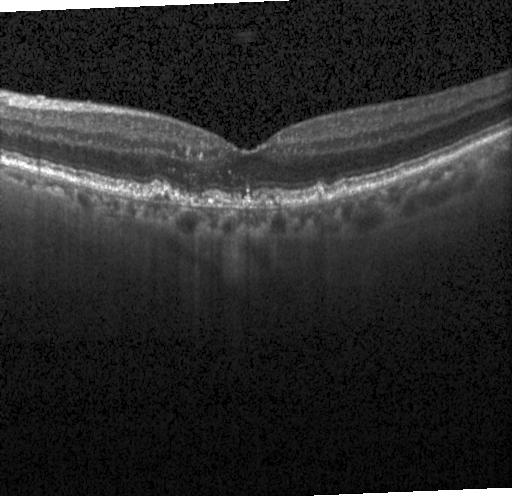
Spectral-domain OCT; Heidelberg Spectralis OCT system; retinal OCT cross-section — Finding: sub-RPE drusenoid deposits.